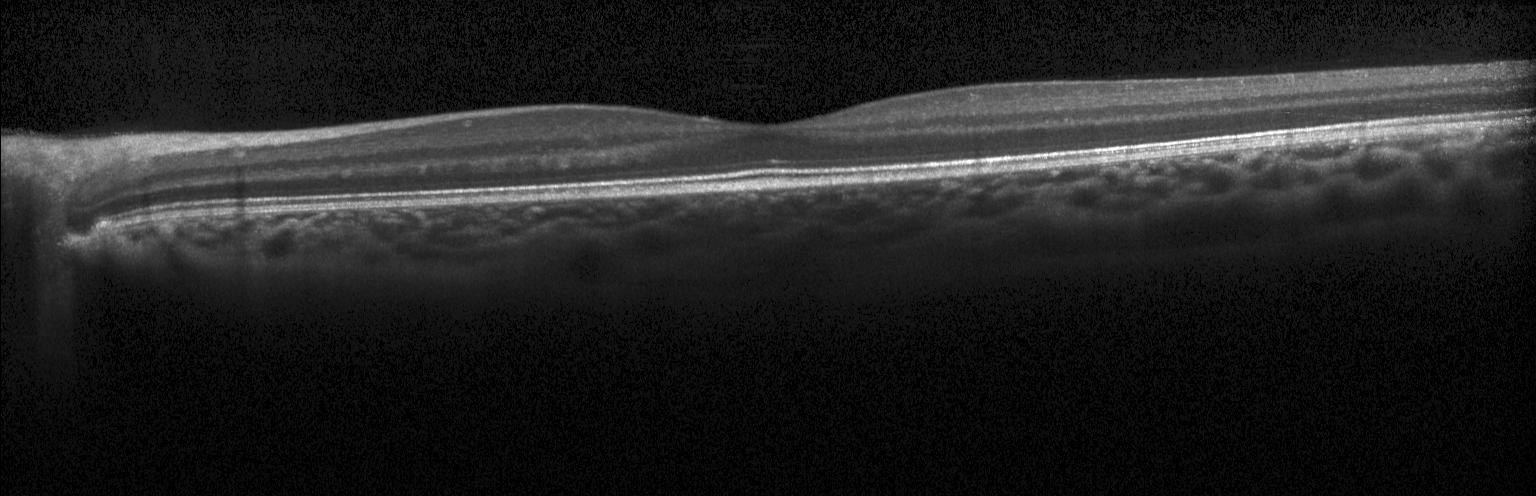 OCT line scan. SD-OCT. Fovea-centered. Dx: no CNV, DME, or drusen.